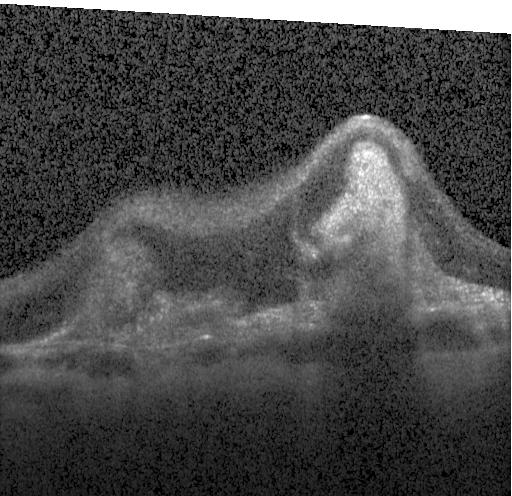
Retinal OCT B-scan; acquired on a Heidelberg Spectralis; macular scan; spectral-domain optical coherence tomography. Choroidal neovascularization.